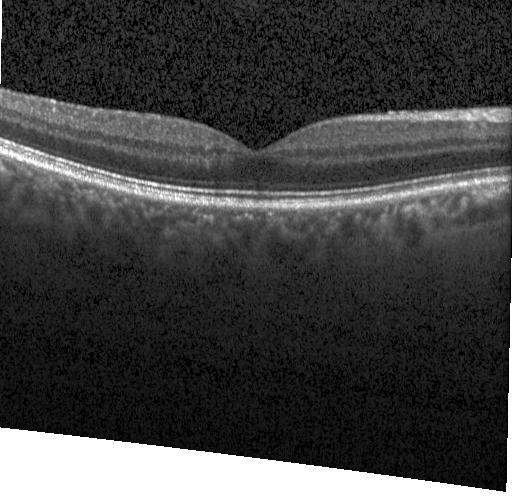 OCT B-scan. Through the macula. Spectral-domain optical coherence tomography. Heidelberg Spectralis.
Diagnosis: no evidence of choroidal neovascularization, diabetic macular edema, or drusen.